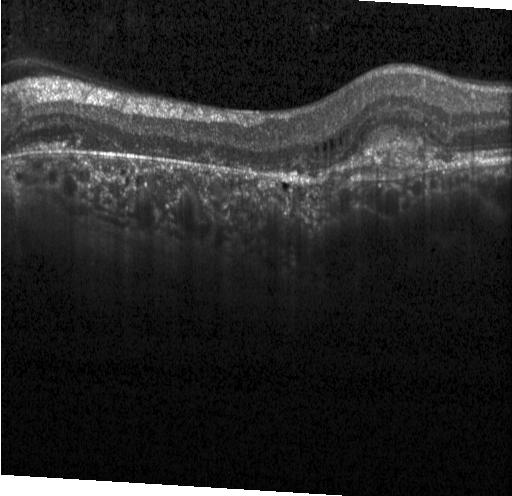
Optical coherence tomography scan; Heidelberg Spectralis OCT system; SD-OCT; horizontal scan through the fovea
OCT finding: CNV.